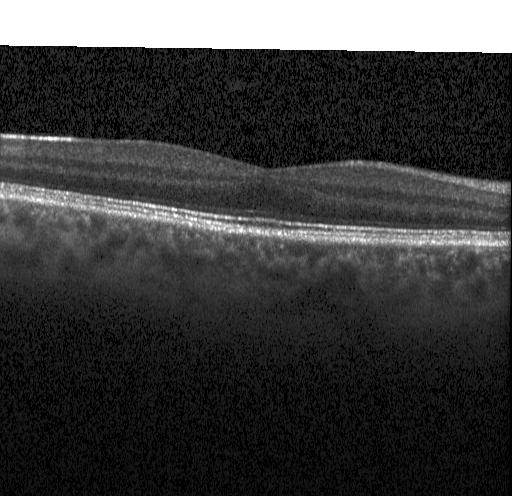 Retinal OCT cross-section showing no choroidal neovascularization, diabetic macular edema, or drusen.